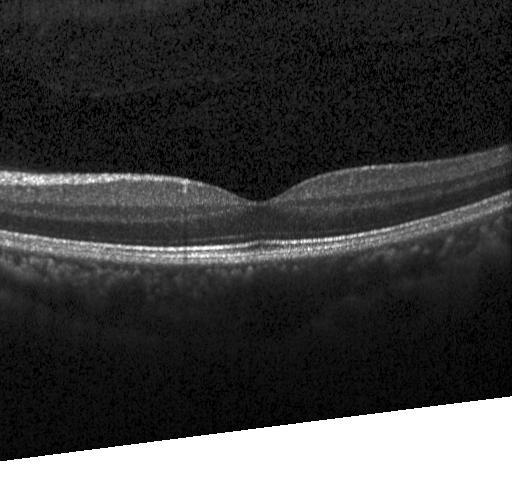
Impression: neither choroidal neovascularization, diabetic macular edema, nor drusen.